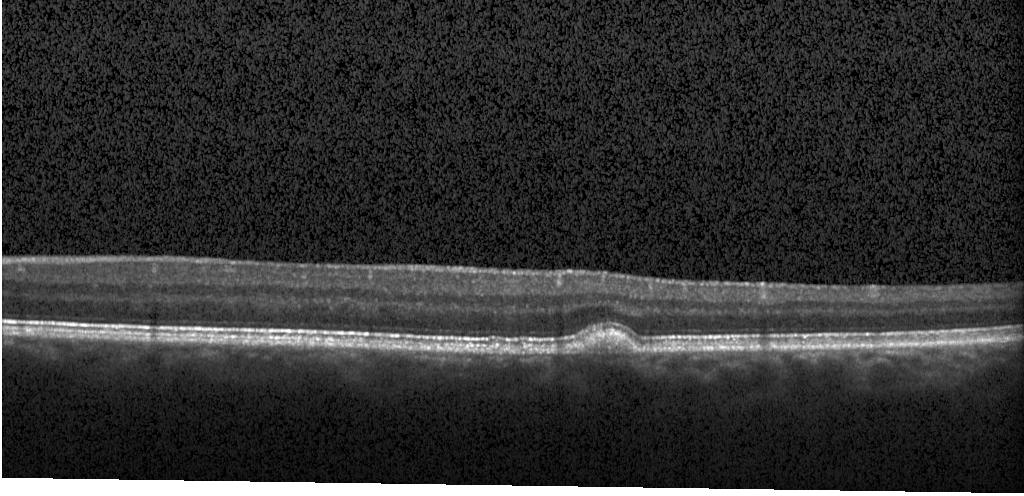
OCT B-scan. This B-scan demonstrates drusen.